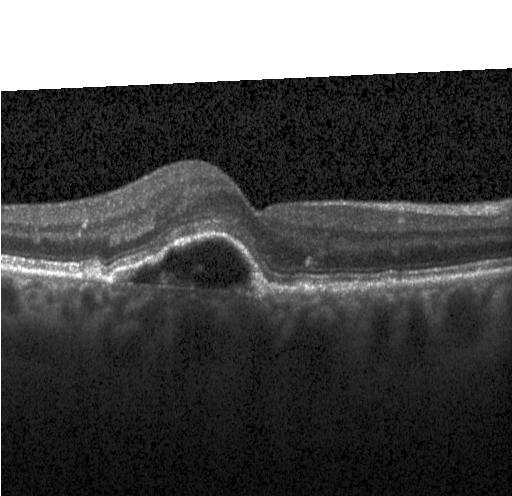 Dx: a choroidal neovascular membrane.